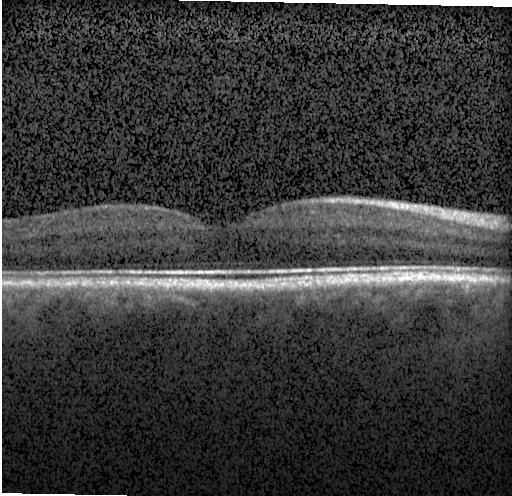

Heidelberg Spectralis; OCT line scan; spectral-domain OCT; centered on the fovea
Finding: no CNV, DME, or drusen.